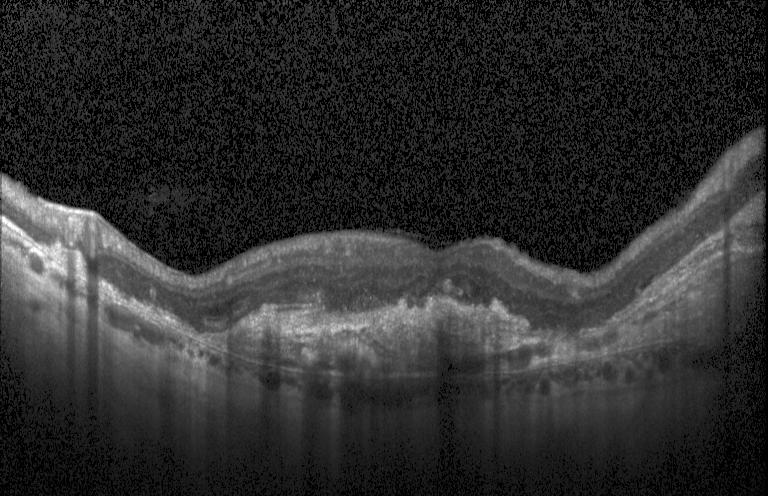

Finding: a choroidal neovascular membrane.